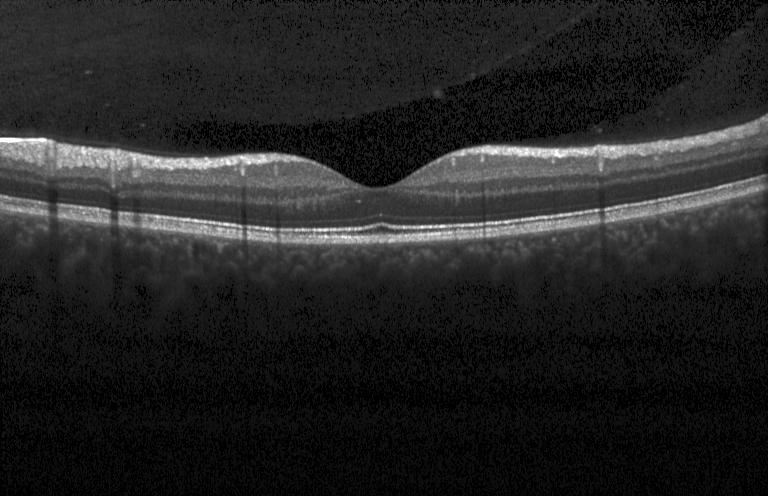
OCT finding: no evidence of choroidal neovascularization, diabetic macular edema, or drusen.